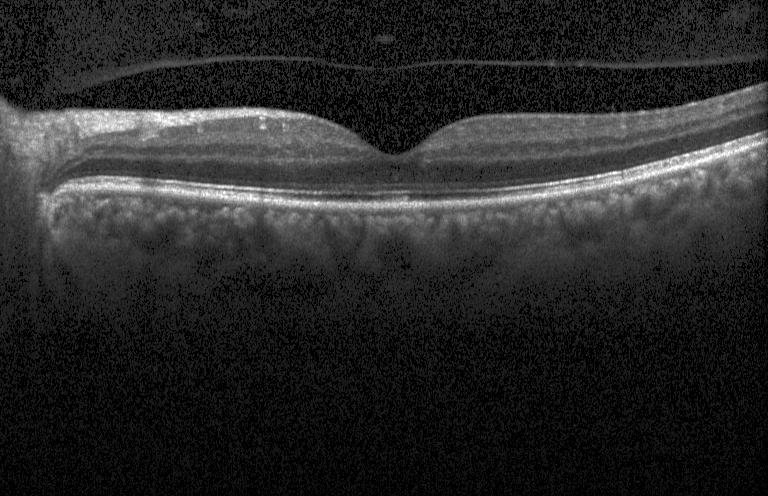 Finding: neither CNV, DME, nor drusen.